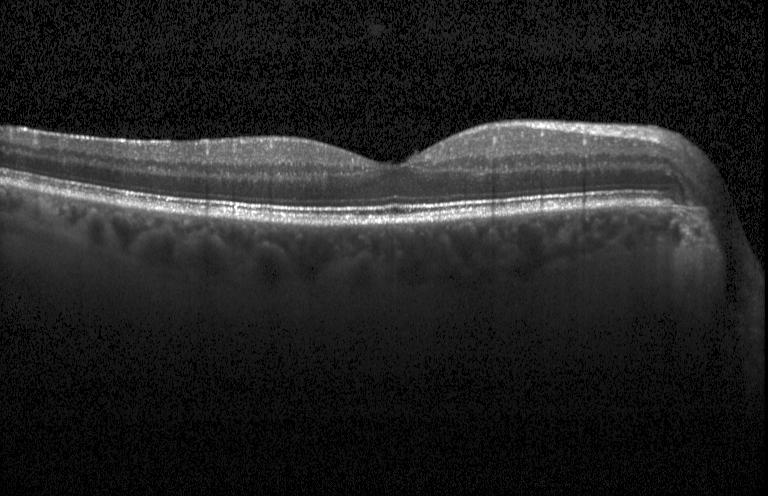
Macular OCT: no evidence of choroidal neovascularization, diabetic macular edema, or drusen.